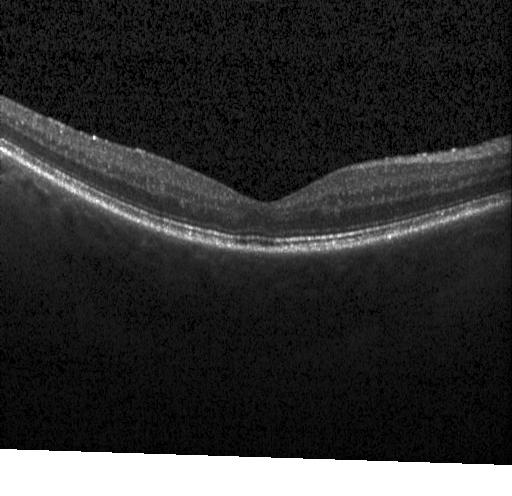

Acquired on a Heidelberg Spectralis, macular scan, spectral-domain OCT, OCT B-scan.
This B-scan demonstrates neither choroidal neovascularization, diabetic macular edema, nor drusen.